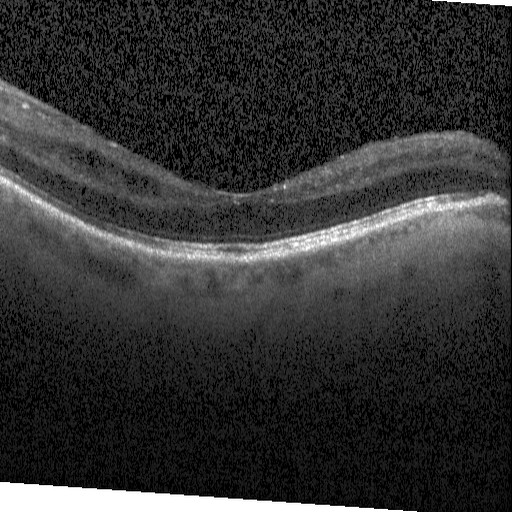

Impression: diabetic macular edema (DME).